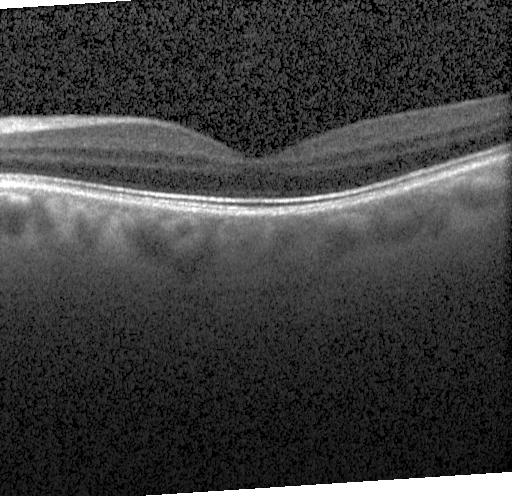

Heidelberg Spectralis. Horizontal scan through the fovea. Spectral-domain OCT. OCT B-scan.
Assessment: no choroidal neovascularization, diabetic macular edema, or drusen.